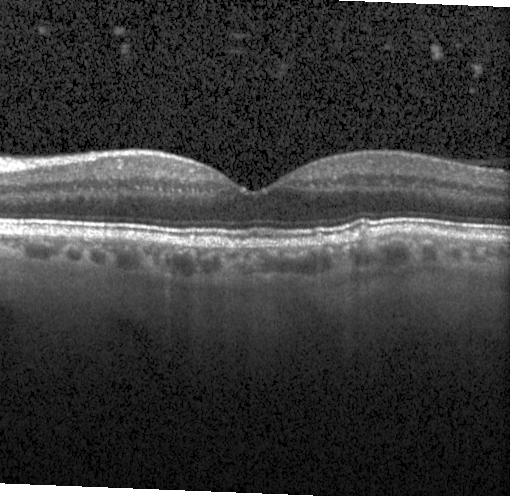

Diagnosis: no evidence of choroidal neovascularization, diabetic macular edema, or drusen.